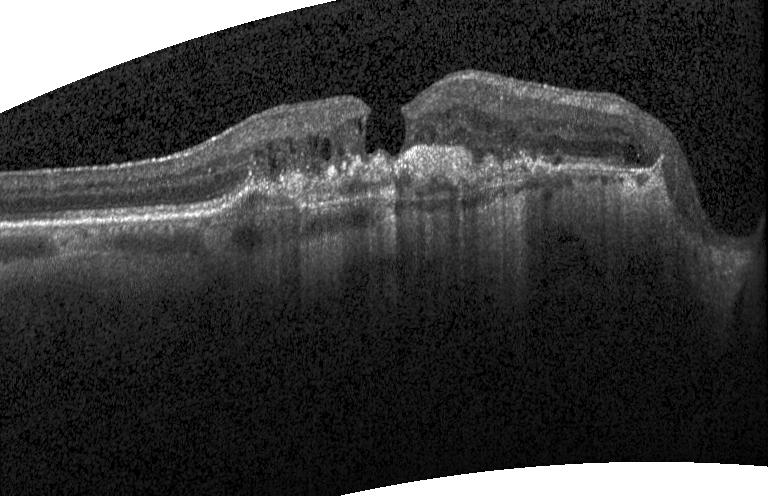 The scan shows choroidal neovascularization.